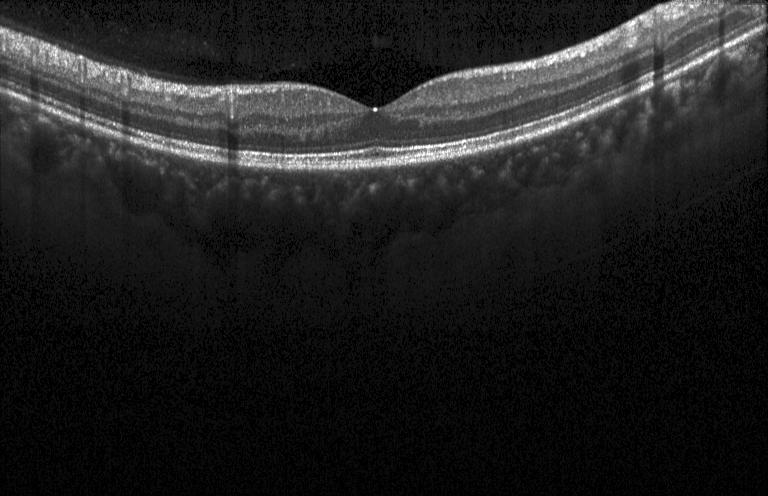
Retinal OCT cross-section. The scan shows no choroidal neovascularization, diabetic macular edema, or drusen.